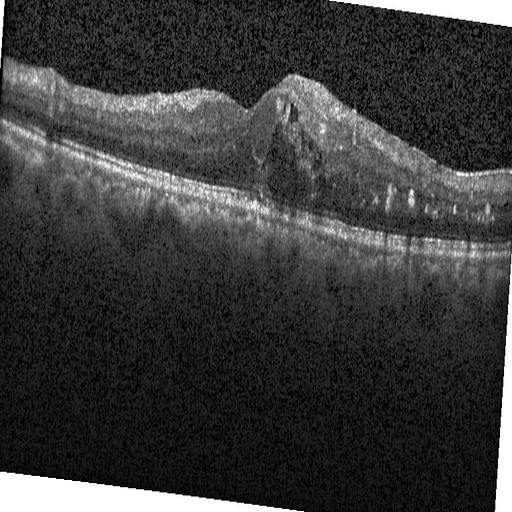

Retinal OCT B-scan · instrument: Heidelberg Spectralis — Diagnosis: DME.